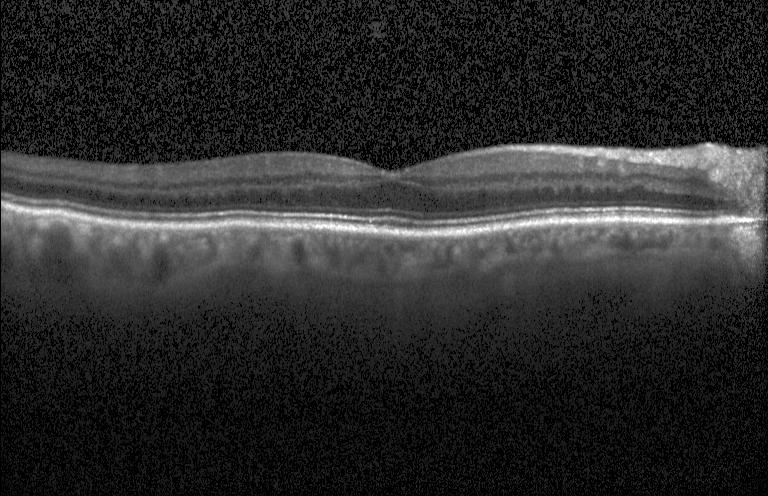

Instrument: Heidelberg Spectralis; spectral-domain OCT; retinal OCT B-scan
This B-scan demonstrates neither choroidal neovascularization, diabetic macular edema, nor drusen.